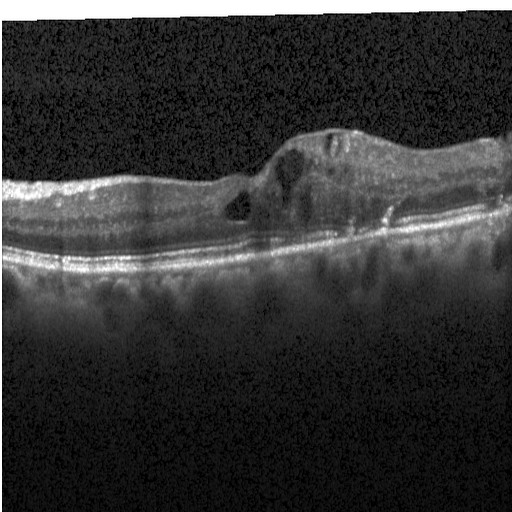
Heidelberg Spectralis. Centered on the fovea. Optical coherence tomography scan.
Diabetic macular edema.